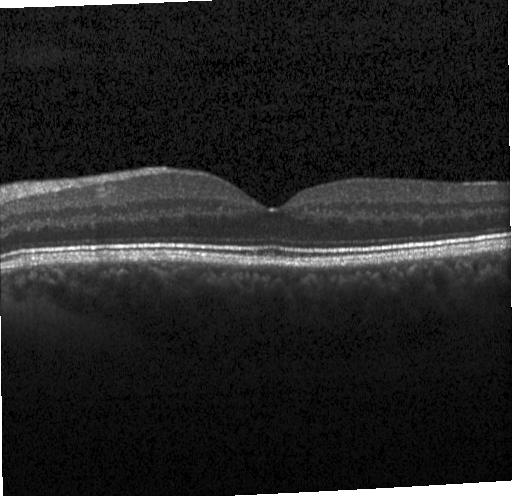
Macular OCT: no evidence of CNV, DME, or drusen.